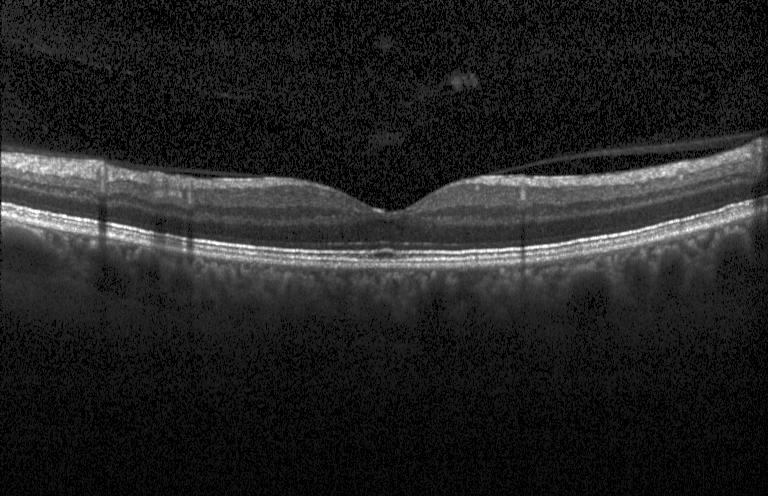 OCT scan showing no evidence of choroidal neovascularization, diabetic macular edema, or drusen.